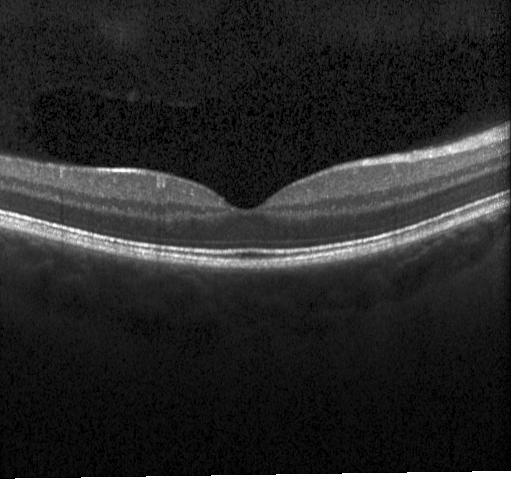
Spectral-domain optical coherence tomography · through the macula · retinal OCT B-scan · Heidelberg Spectralis. Finding: no choroidal neovascularization, no diabetic macular edema, and no drusen.